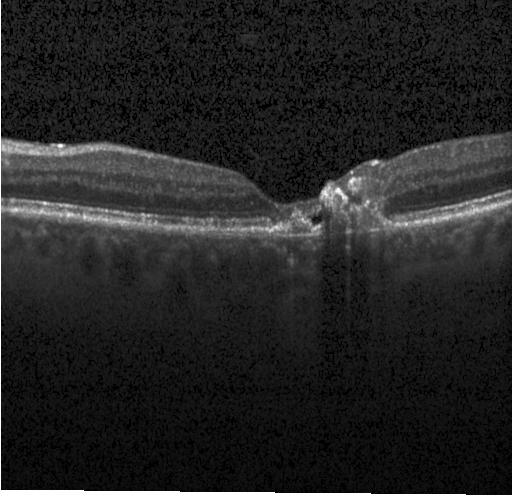
OCT B-scan.
The scan shows a choroidal neovascular membrane.